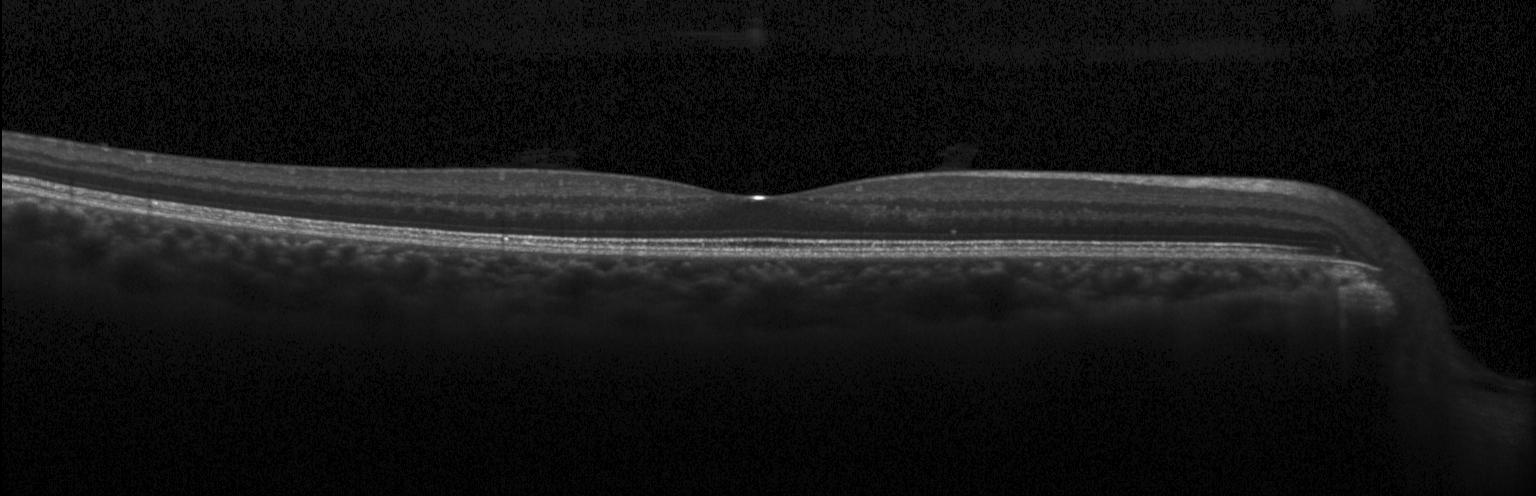

Impression: no choroidal neovascularization, diabetic macular edema, or drusen.